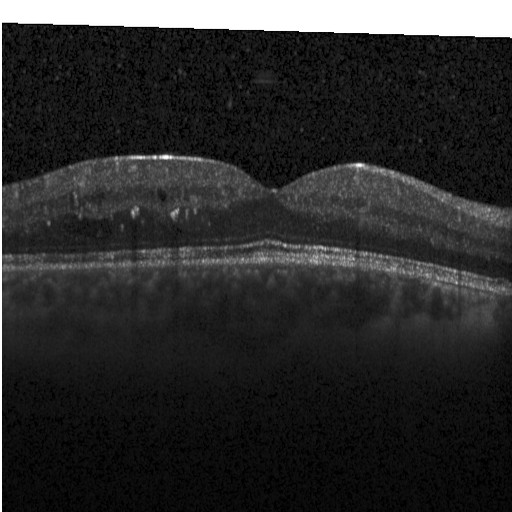

Macular OCT: diabetic macular edema (DME).